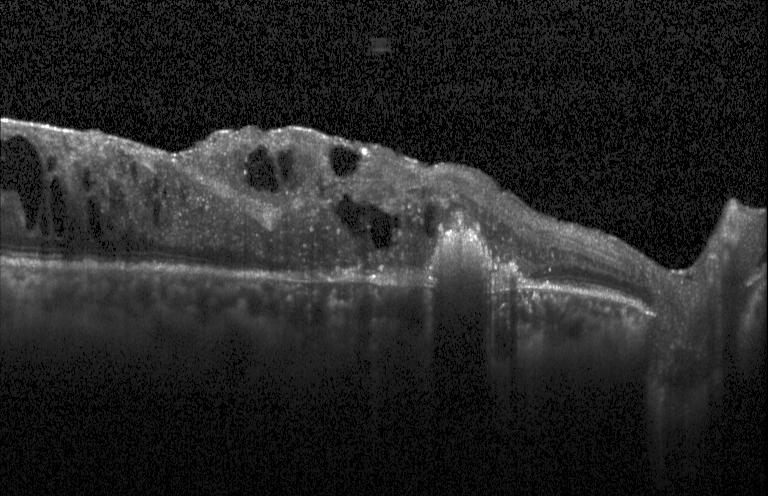
Impression: choroidal neovascularization (CNV).